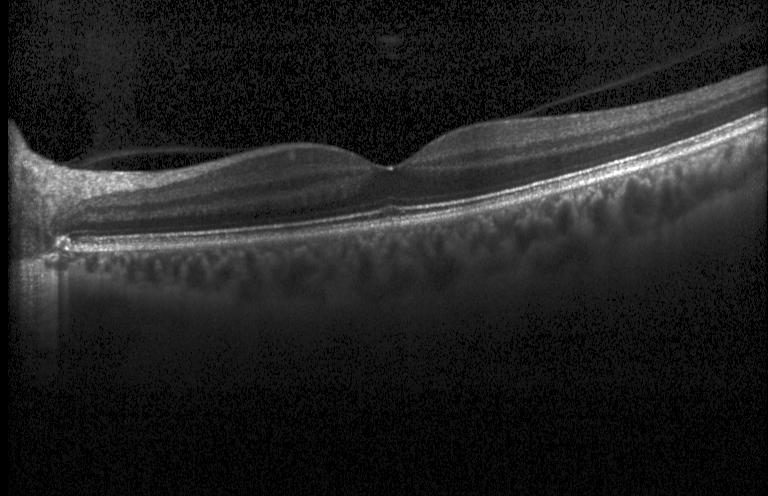 Finding: no evidence of choroidal neovascularization, diabetic macular edema, or drusen.